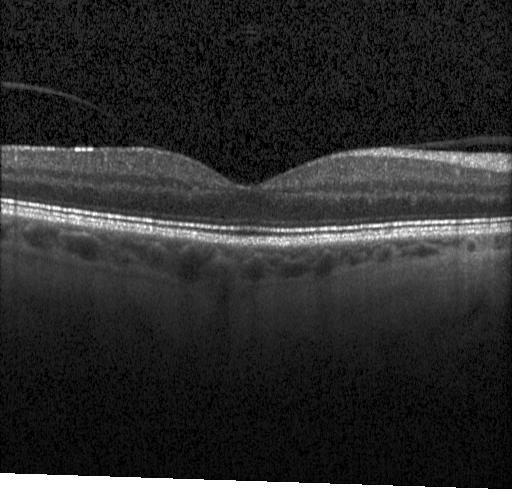
Heidelberg Spectralis; spectral-domain optical coherence tomography; OCT line scan; centered on the fovea — Macular OCT: neither choroidal neovascularization, diabetic macular edema, nor drusen.